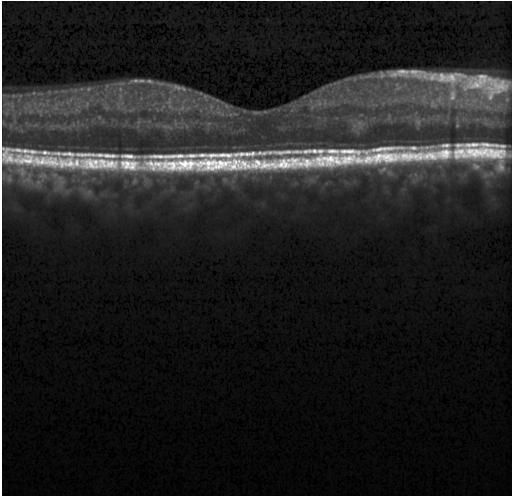
Dx: no CNV, DME, or drusen.